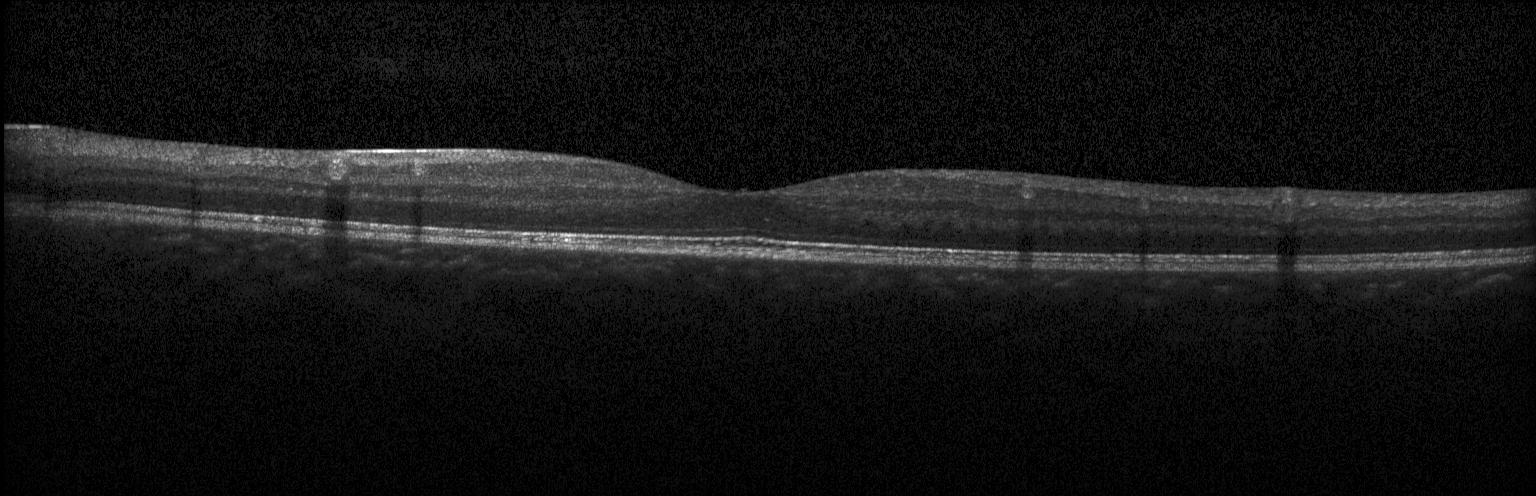
Finding: neither CNV, DME, nor drusen.